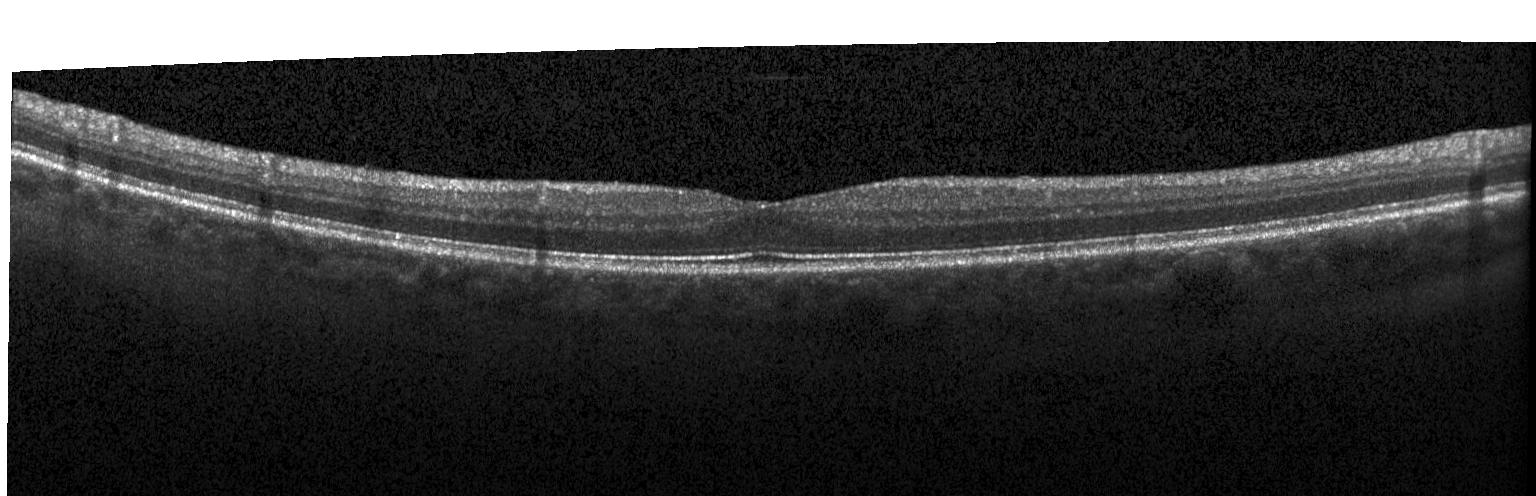

Diagnosis: no choroidal neovascularization, diabetic macular edema, or drusen.